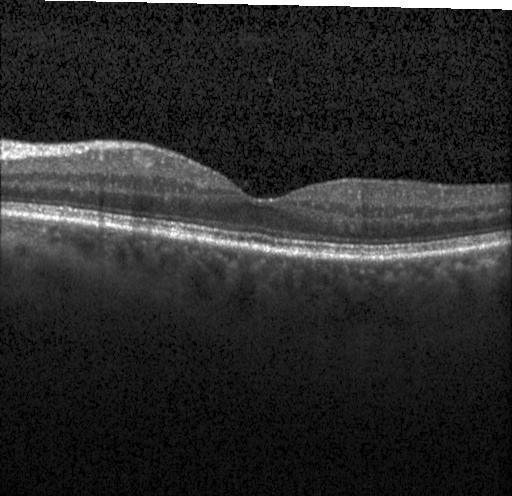

Heidelberg Spectralis, SD-OCT, optical coherence tomography B-scan
Macular OCT: neither CNV, DME, nor drusen.